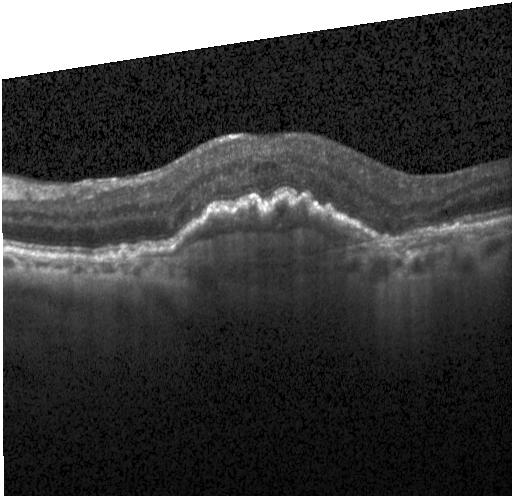
Horizontal scan through the fovea · spectral-domain OCT · OCT line scan
Finding: a choroidal neovascular membrane.